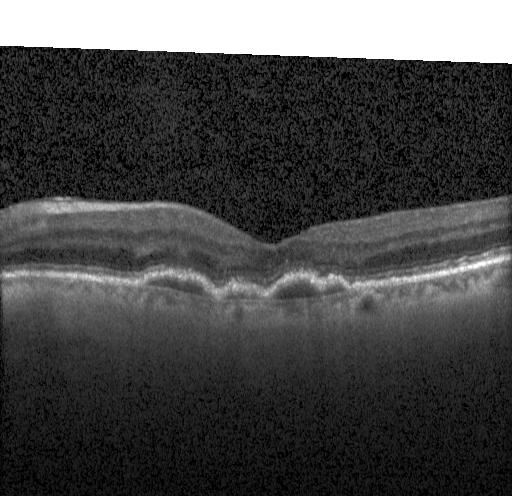 Dx: a choroidal neovascular membrane.